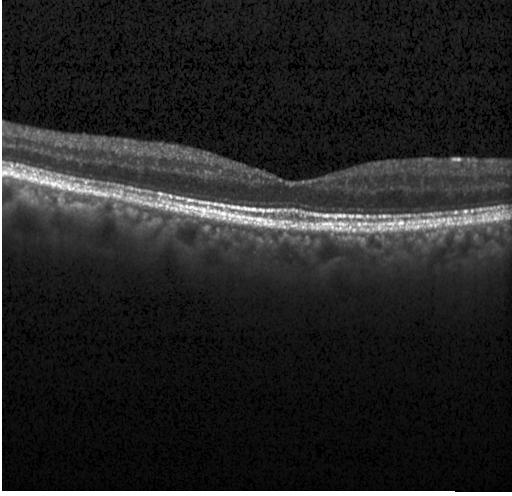
OCT finding: no choroidal neovascularization, no diabetic macular edema, and no drusen.